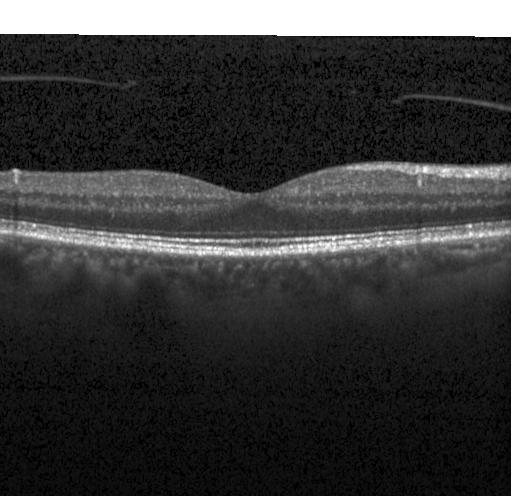

Finding: neither CNV, DME, nor drusen.